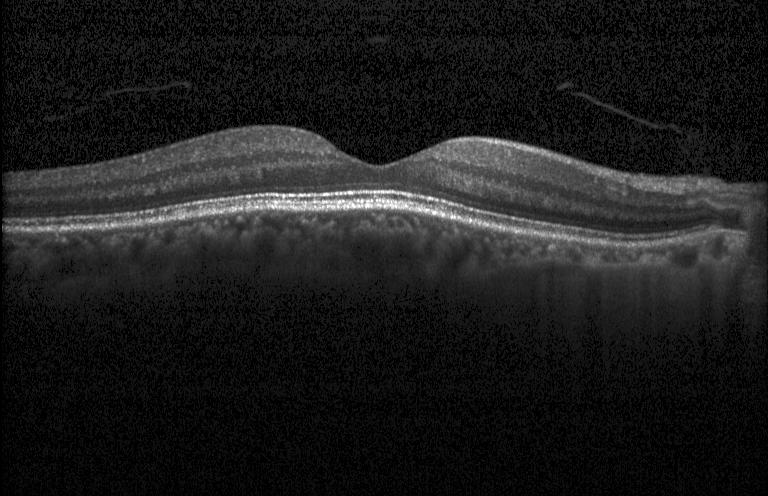 Macular OCT: no evidence of CNV, DME, or drusen.